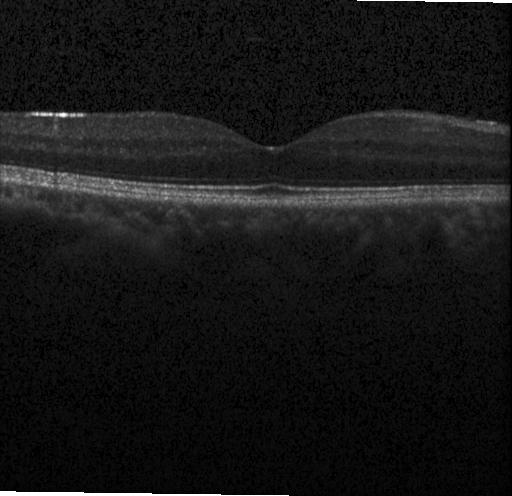 Acquired on a Heidelberg Spectralis. SD-OCT. Optical coherence tomography scan — Impression: neither choroidal neovascularization, diabetic macular edema, nor drusen.